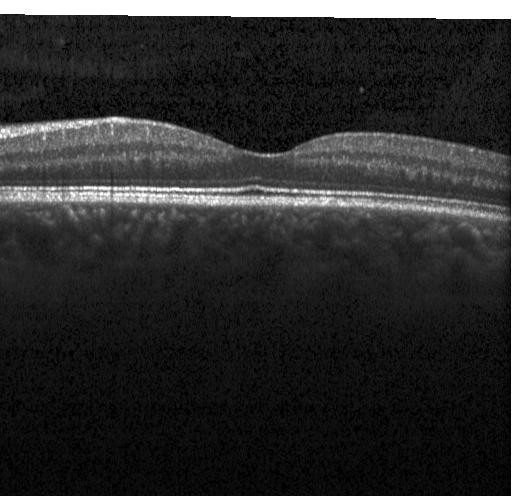

Dx: no evidence of choroidal neovascularization, diabetic macular edema, or drusen.